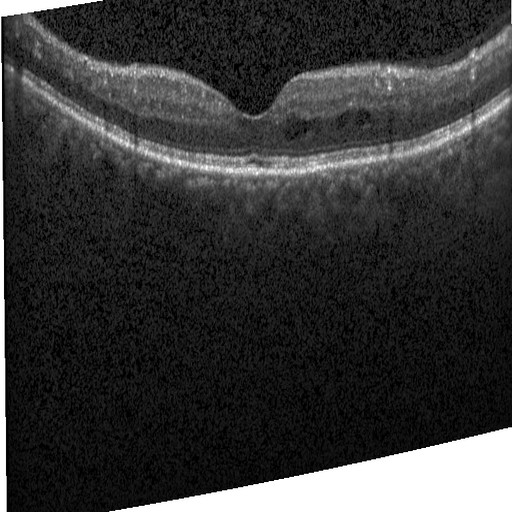
Impression: diabetic macular edema.